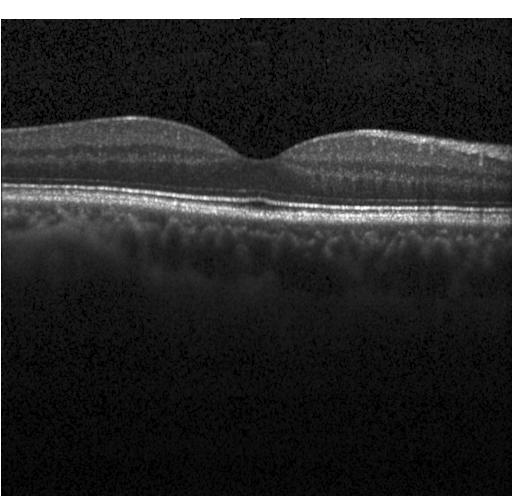 Optical coherence tomography B-scan · Heidelberg Spectralis · spectral-domain optical coherence tomography. Finding: no choroidal neovascularization, no diabetic macular edema, and no drusen.